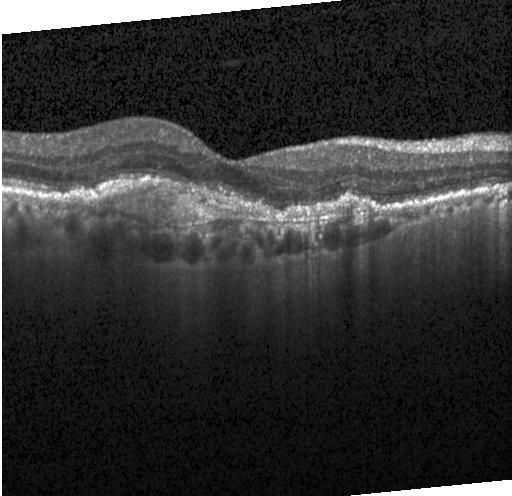
Horizontal scan through the fovea · optical coherence tomography B-scan — Dx: choroidal neovascularization.